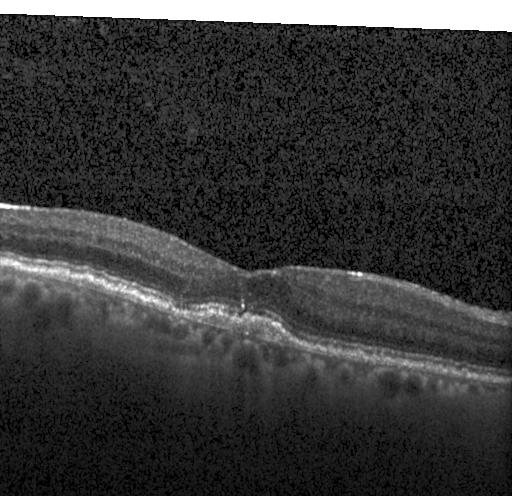

Spectral-domain OCT B-scan: a choroidal neovascular membrane.